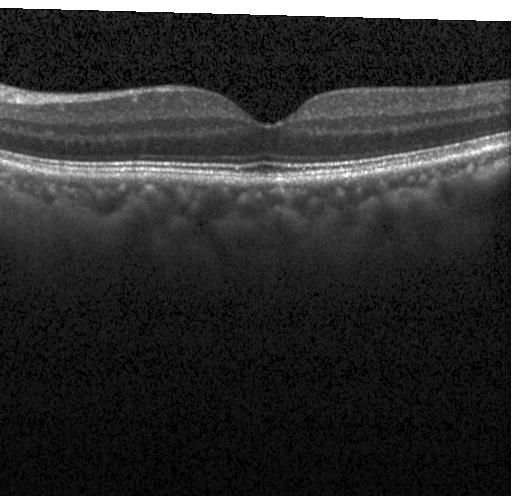
Horizontal scan through the fovea; Heidelberg Spectralis OCT system; optical coherence tomography scan; SD-OCT. No CNV, no DME, and no drusen.